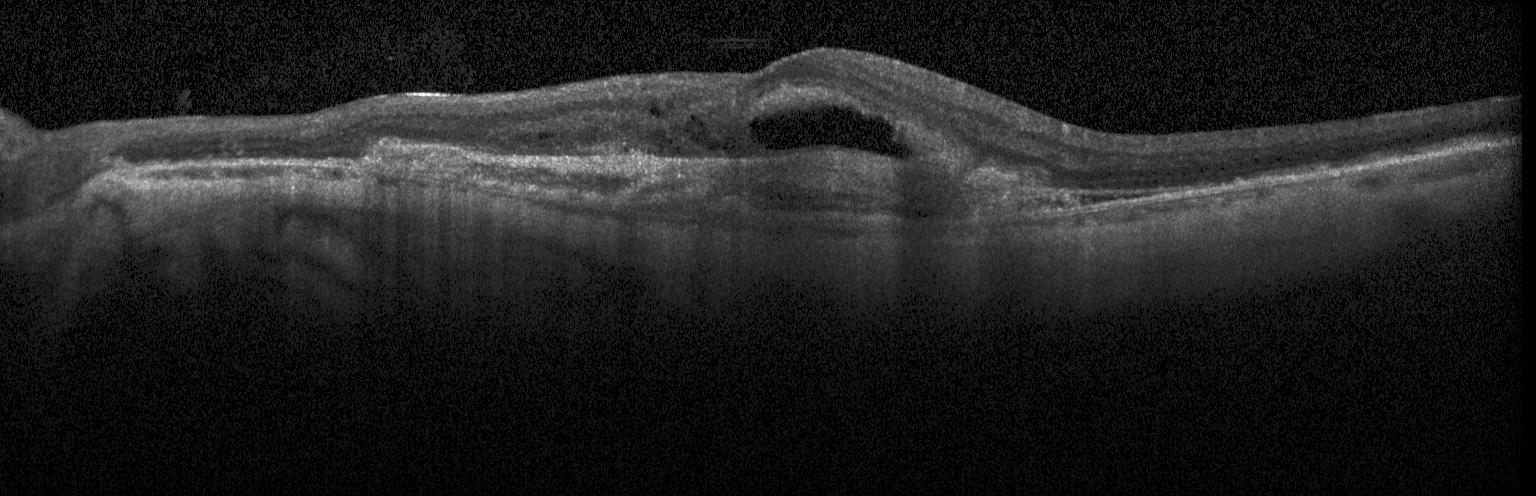 SD-OCT; Heidelberg Spectralis; through the macula; optical coherence tomography B-scan.
A choroidal neovascular membrane.